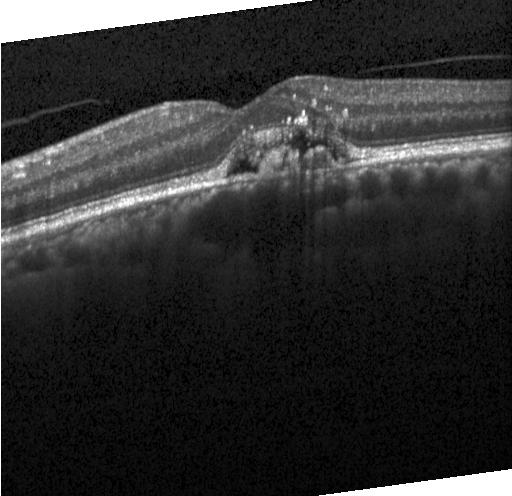 Optical coherence tomography scan. Finding: CNV.